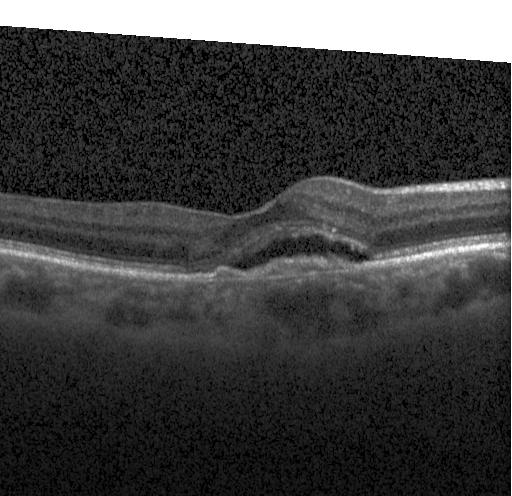 OCT line scan; through the macula; instrument: Heidelberg Spectralis; SD-OCT. This B-scan demonstrates a choroidal neovascular membrane.